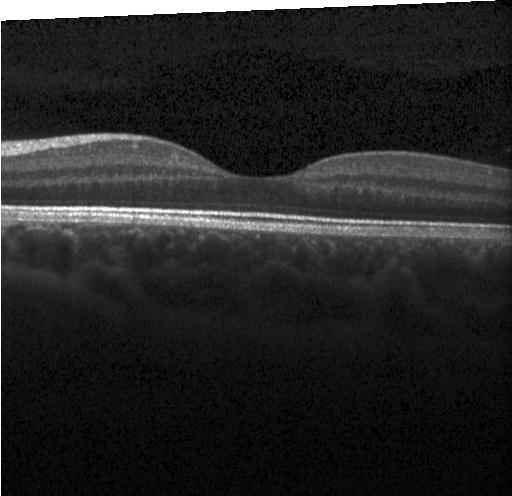

Optical coherence tomography B-scan — Diagnosis: no evidence of choroidal neovascularization, diabetic macular edema, or drusen.